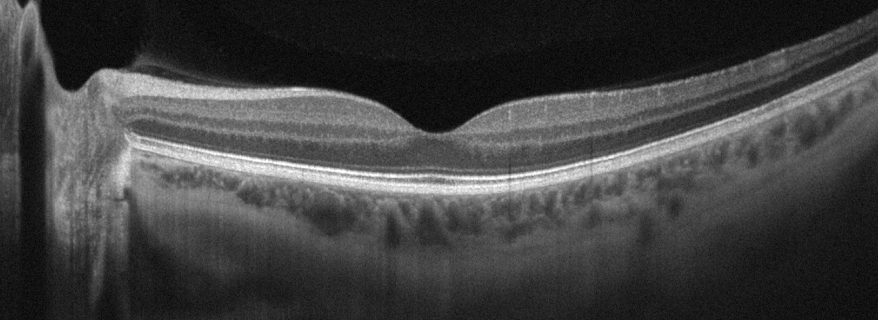

Retinal OCT B-scan. Finding: no AMD, DME, ERM, RAO, RVO, or VID.